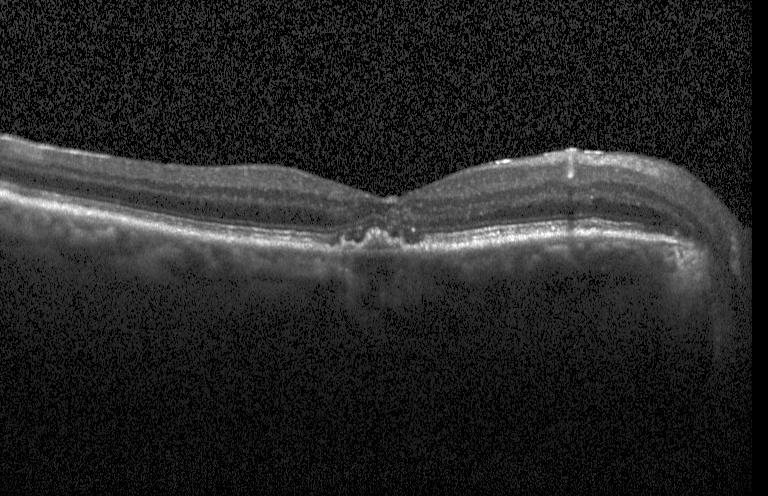
Optical coherence tomography scan. Impression: CNV.